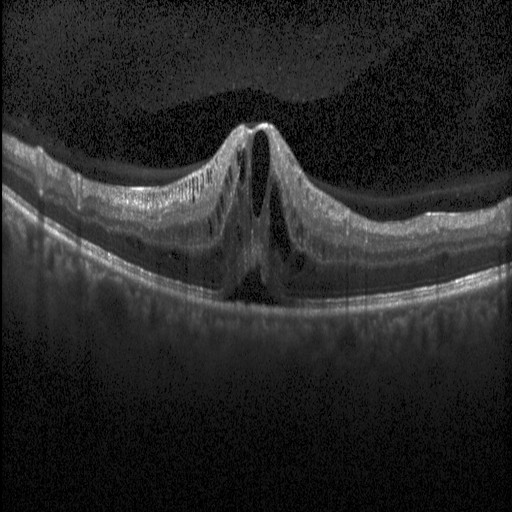 Impression: DME.